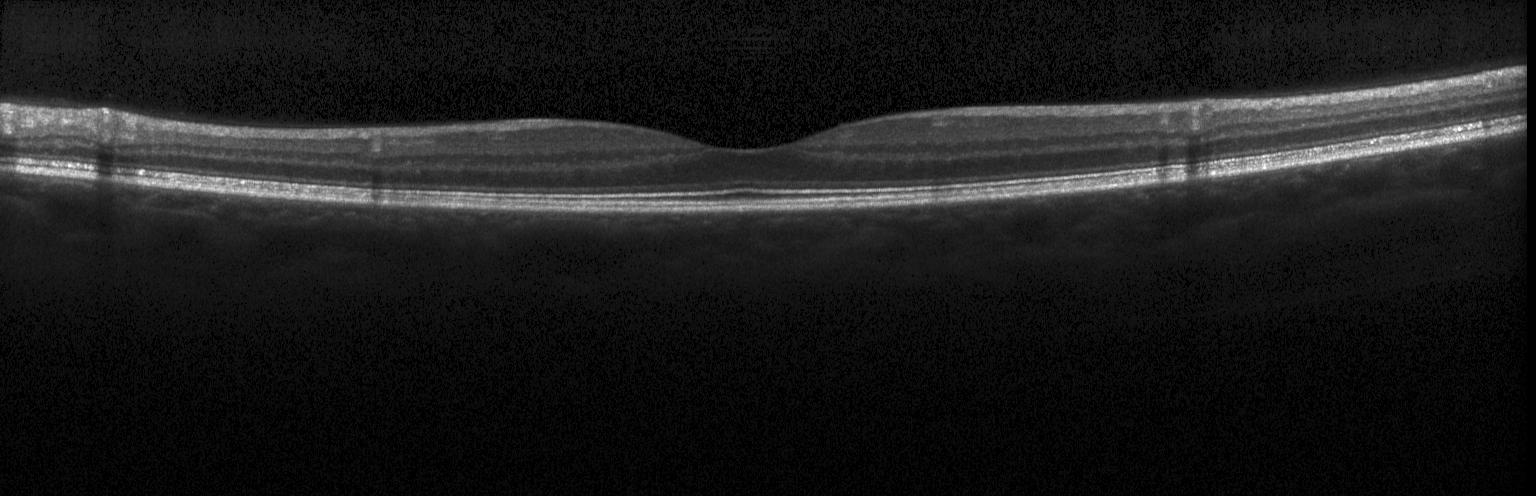

Macular scan · SD-OCT · Heidelberg Spectralis · OCT B-scan — OCT finding: neither choroidal neovascularization, diabetic macular edema, nor drusen.